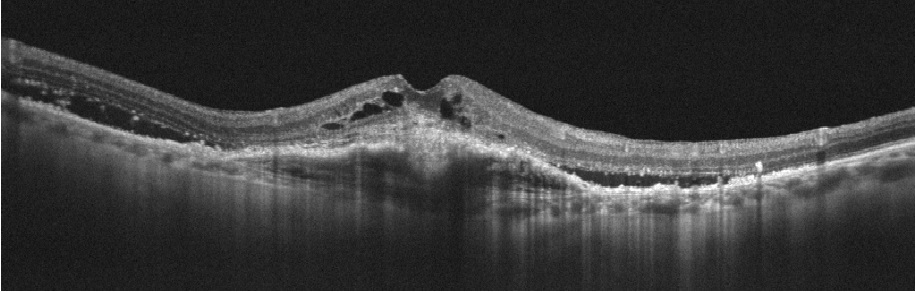 Optical coherence tomography scan — Finding: age-related macular degeneration.